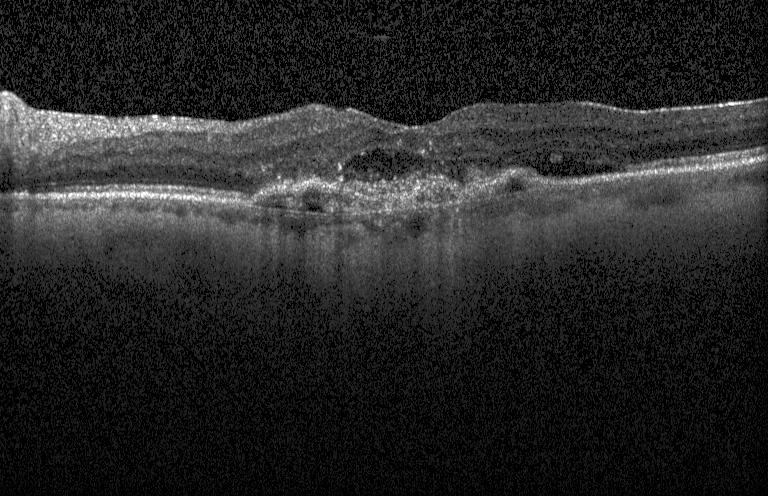
Macular OCT: a choroidal neovascular membrane.